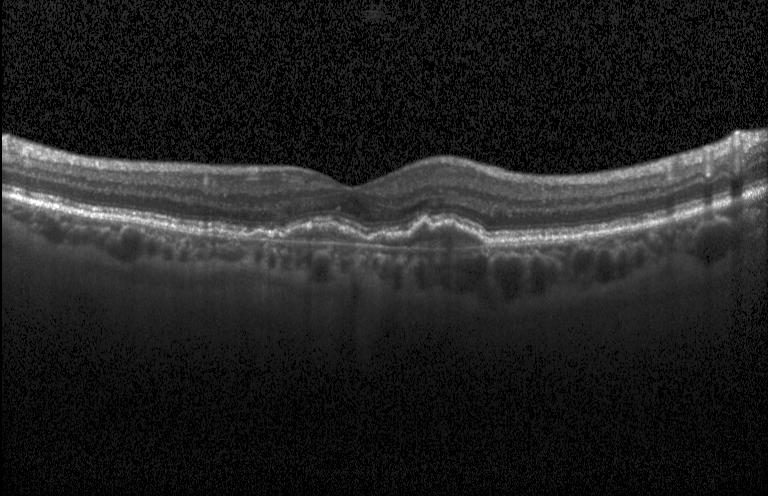

OCT finding: choroidal neovascularization.